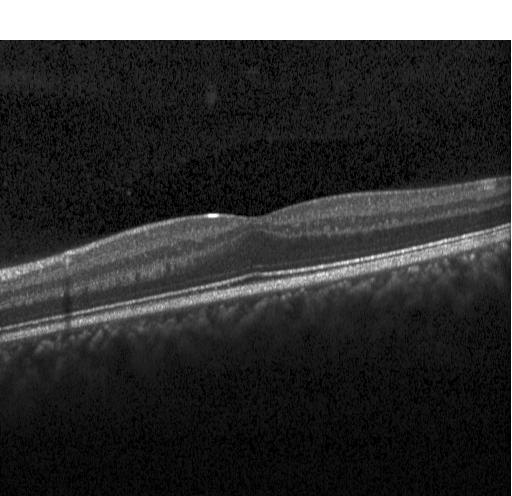 Retinal OCT B-scan — Diagnosis: no CNV, no DME, and no drusen.